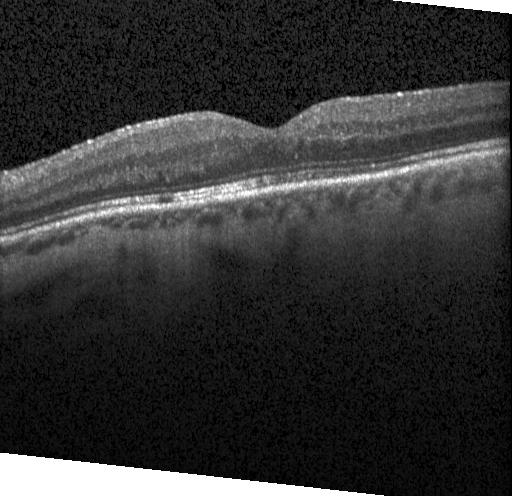

Acquired on a Heidelberg Spectralis · spectral-domain OCT · OCT B-scan · centered on the fovea. Dx: no CNV, no DME, and no drusen.